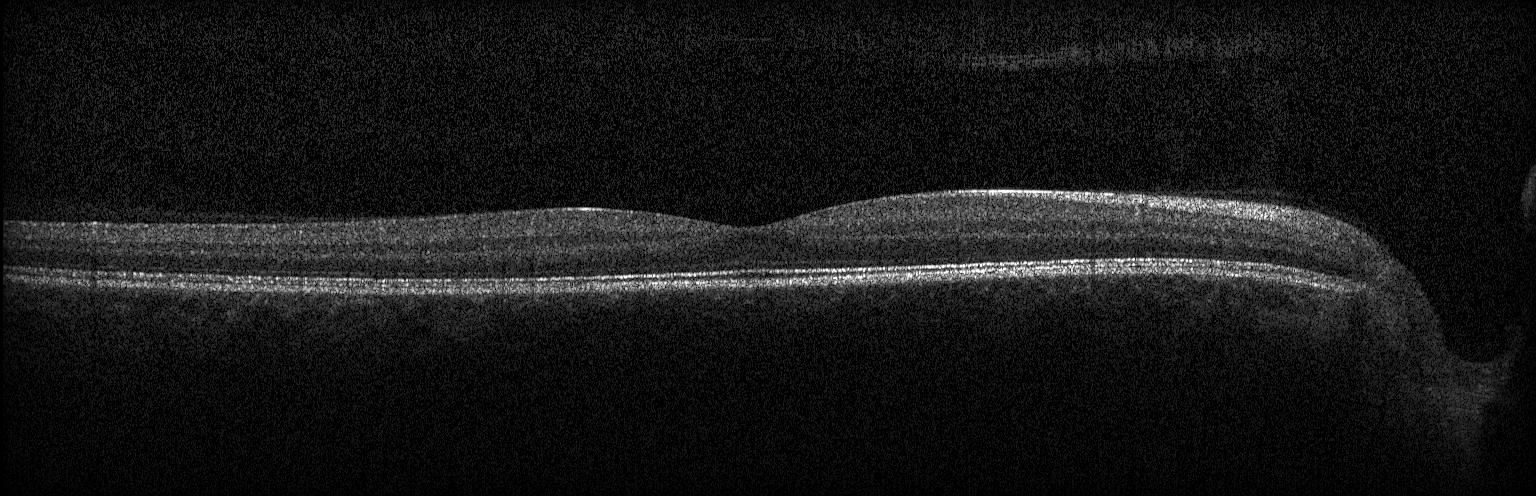 Instrument: Heidelberg Spectralis. Retinal OCT cross-section — Finding: no choroidal neovascularization, no diabetic macular edema, and no drusen.